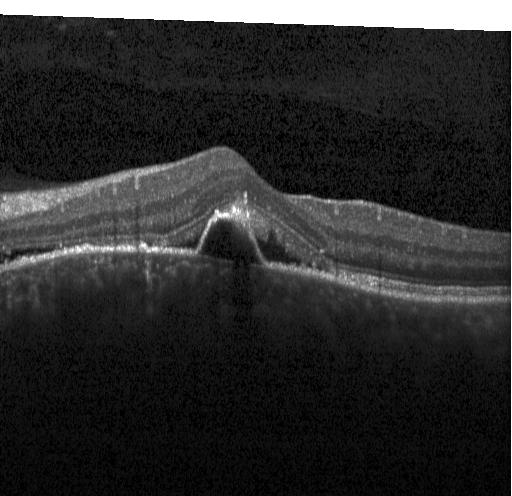
Impression: choroidal neovascularization.